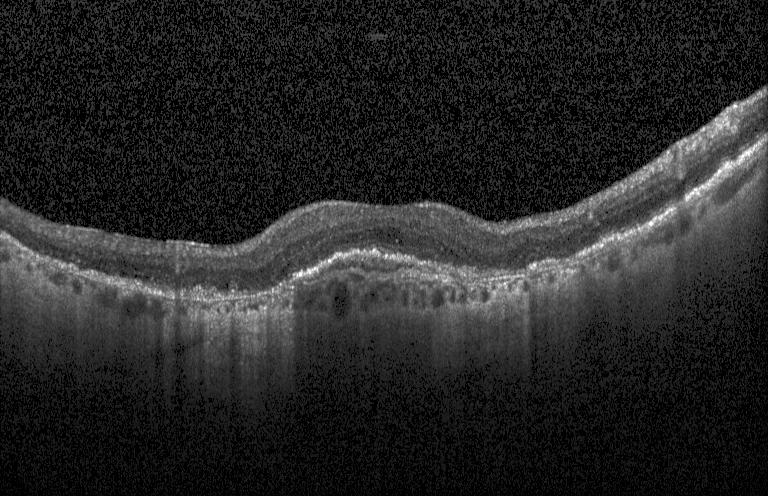

Finding: CNV.